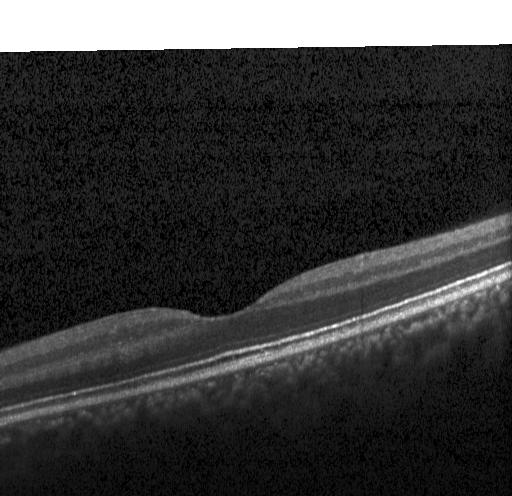

Retinal OCT B-scan; Heidelberg Spectralis. This B-scan demonstrates neither choroidal neovascularization, diabetic macular edema, nor drusen.